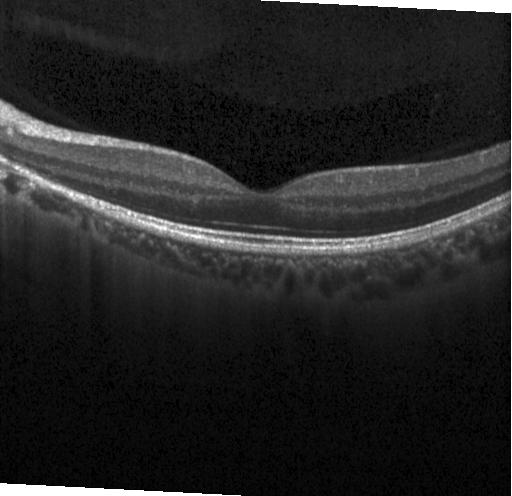 Horizontal scan through the fovea · SD-OCT · Heidelberg Spectralis · retinal OCT B-scan — The scan shows no choroidal neovascularization, no diabetic macular edema, and no drusen.